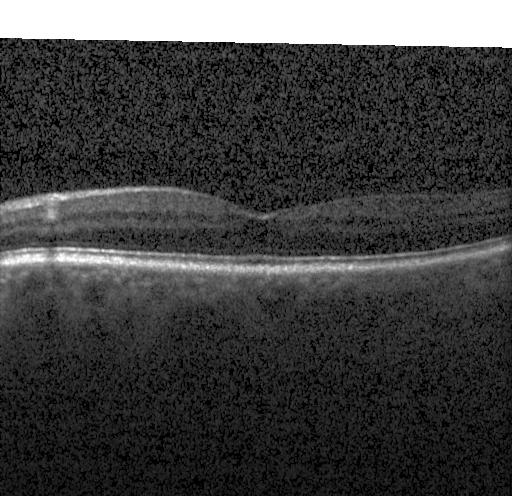
Retinal OCT cross-section showing no evidence of choroidal neovascularization, diabetic macular edema, or drusen.